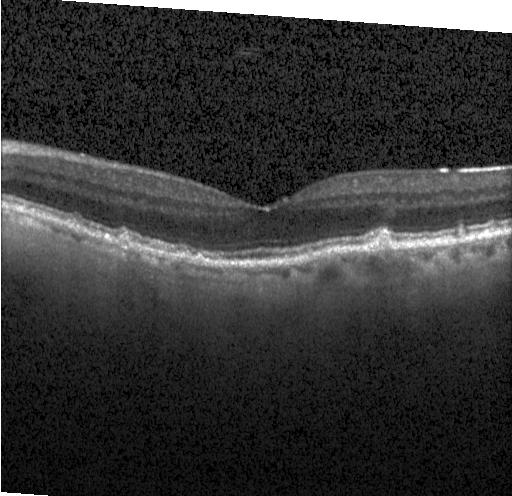
Optical coherence tomography B-scan, SD-OCT.
This B-scan demonstrates multiple drusen.